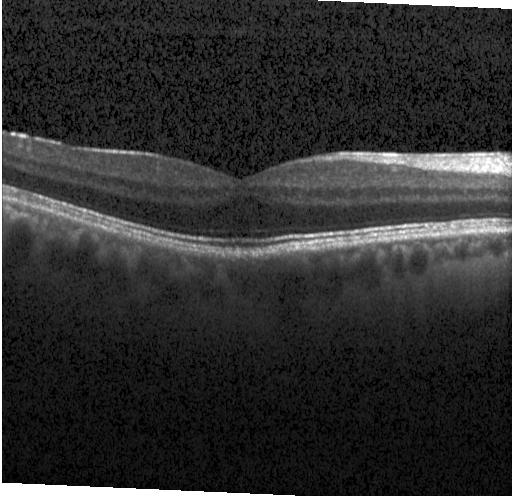
Retinal OCT cross-section, SD-OCT, horizontal scan through the fovea. No choroidal neovascularization, no diabetic macular edema, and no drusen.